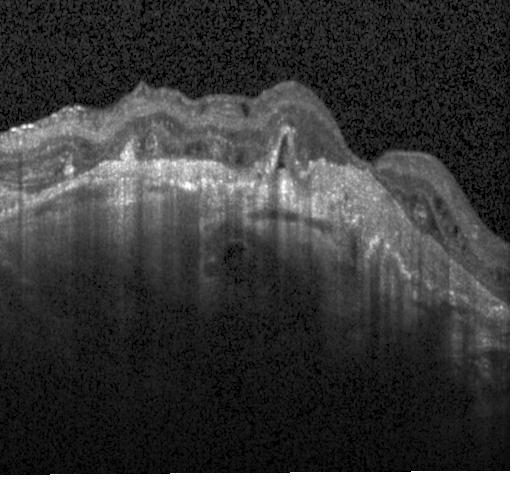 OCT B-scan. Dx: choroidal neovascularization (CNV).